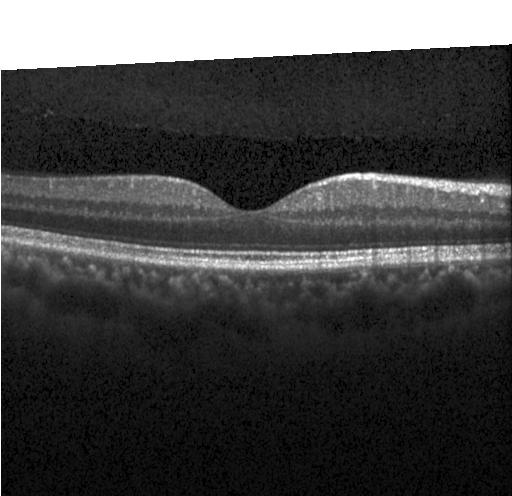 Spectral-domain OCT B-scan: no choroidal neovascularization, diabetic macular edema, or drusen.